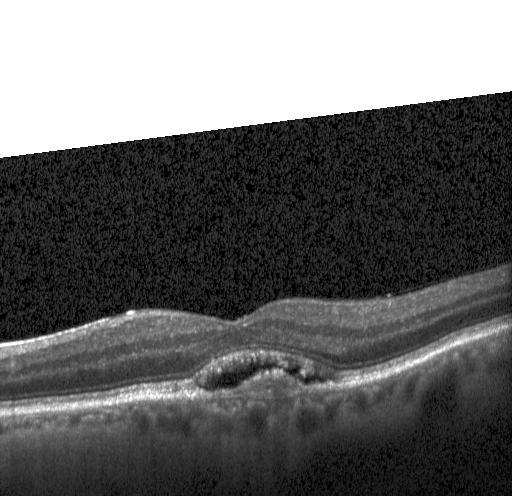
Optical coherence tomography scan.
Finding: choroidal neovascularization.